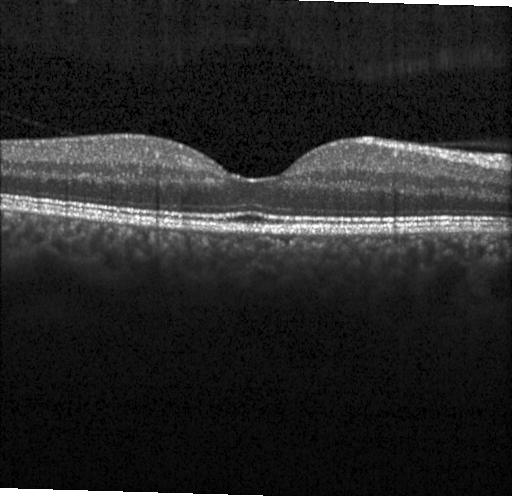

Fovea-centered · retinal OCT cross-section · spectral-domain OCT · instrument: Heidelberg Spectralis — Finding: no choroidal neovascularization, no diabetic macular edema, and no drusen.